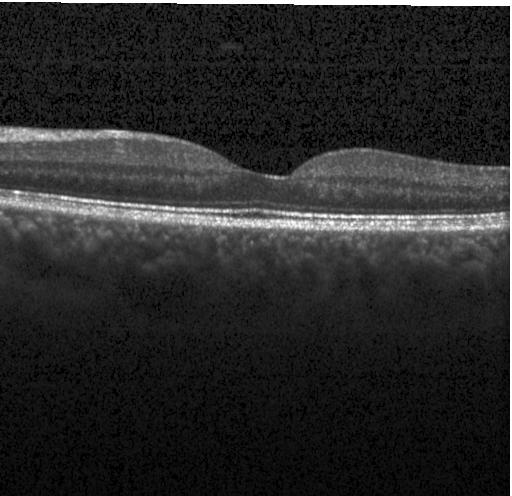 Retinal OCT cross-section showing no evidence of choroidal neovascularization, diabetic macular edema, or drusen.